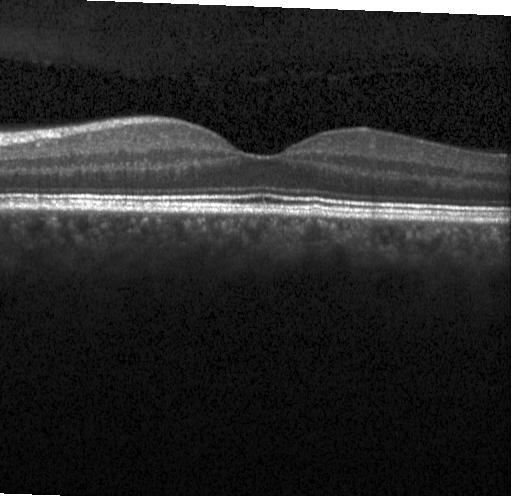
Diagnosis: no CNV, no DME, and no drusen.